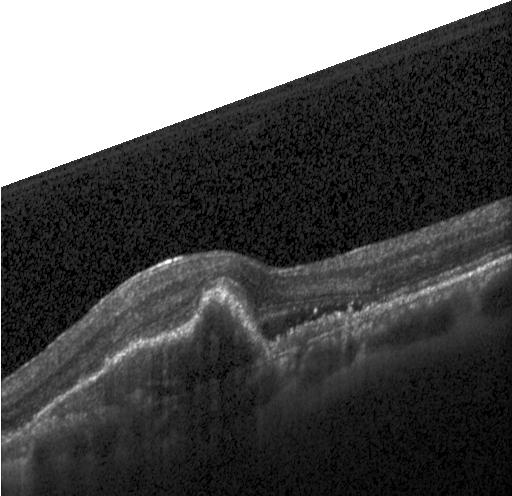
The scan shows a choroidal neovascular membrane.